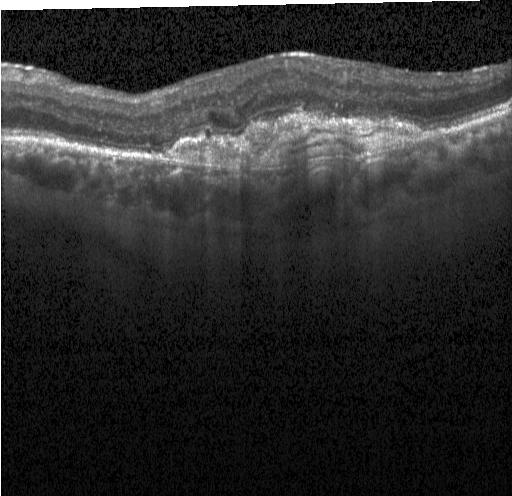
Optical coherence tomography scan — OCT finding: choroidal neovascularization.